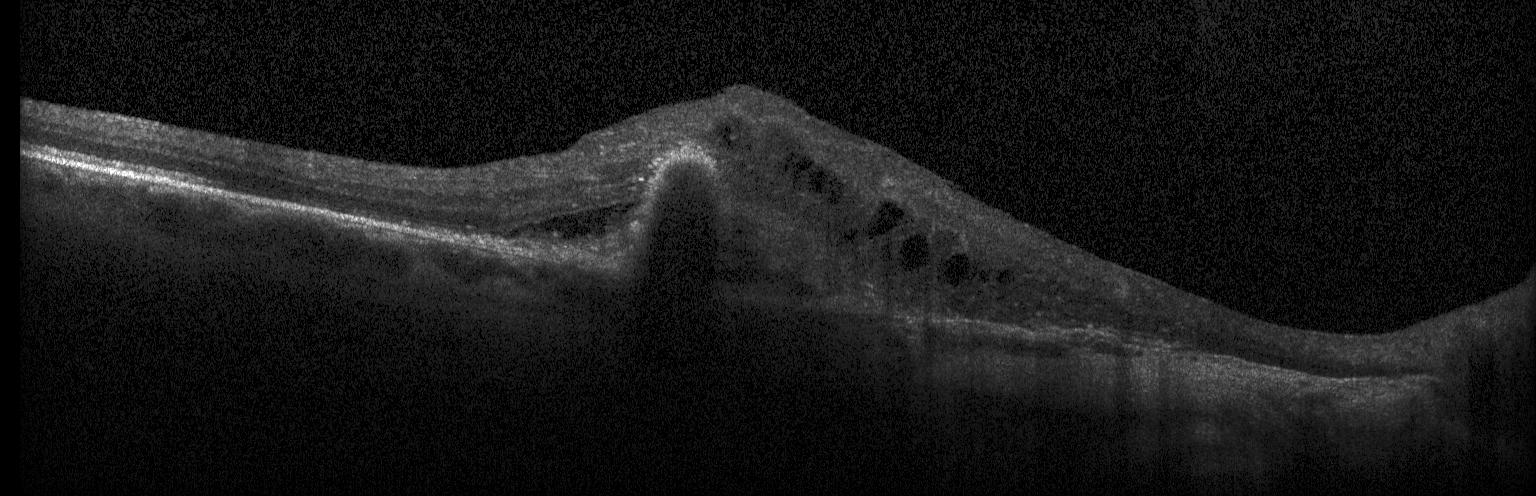
Horizontal scan through the fovea · optical coherence tomography B-scan. Finding: choroidal neovascularization.